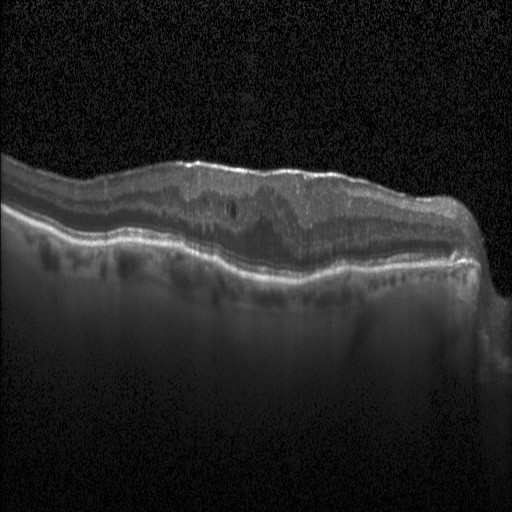

Macular scan; Heidelberg Spectralis; SD-OCT; optical coherence tomography B-scan
OCT finding: diabetic macular edema (DME).